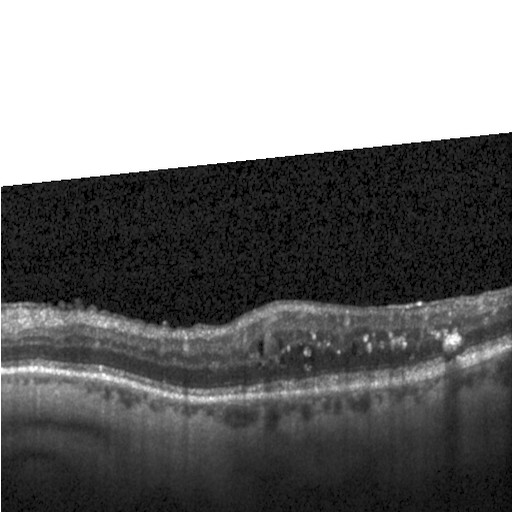 Macular OCT: DME.